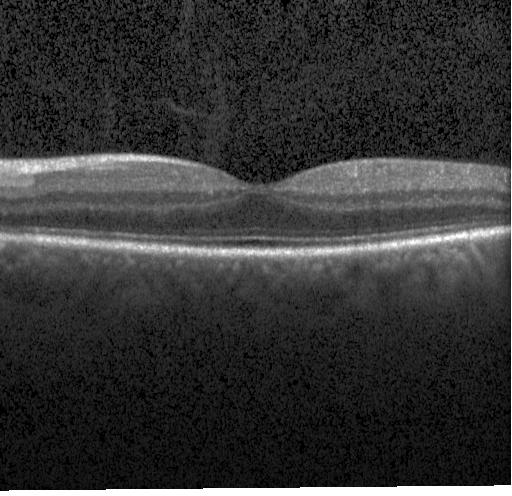

Optical coherence tomography scan
Assessment: no choroidal neovascularization, diabetic macular edema, or drusen.